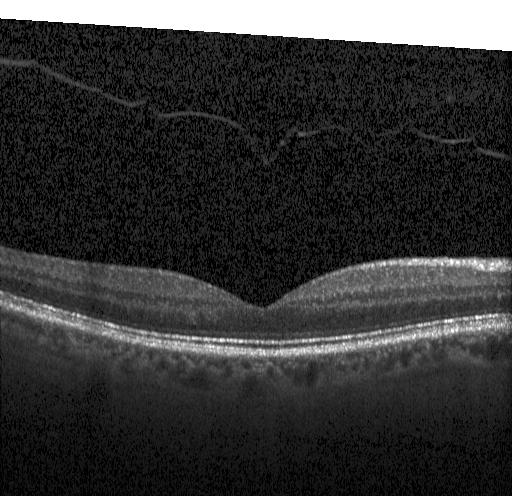

OCT line scan. Dx: no evidence of choroidal neovascularization, diabetic macular edema, or drusen.